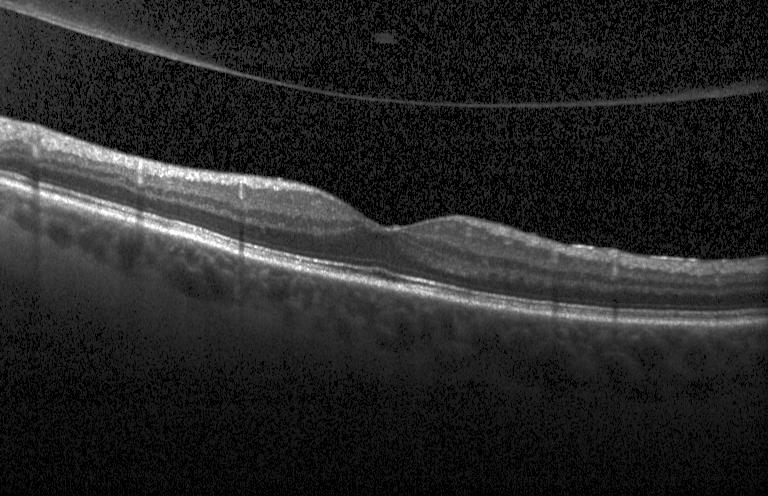

Spectral-domain OCT B-scan: no evidence of CNV, DME, or drusen.